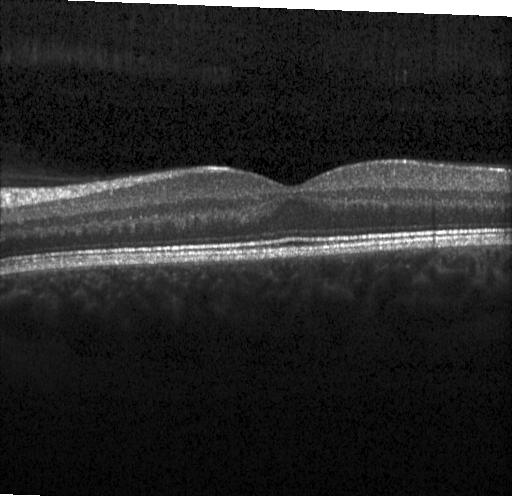
OCT scan showing no choroidal neovascularization, no diabetic macular edema, and no drusen.